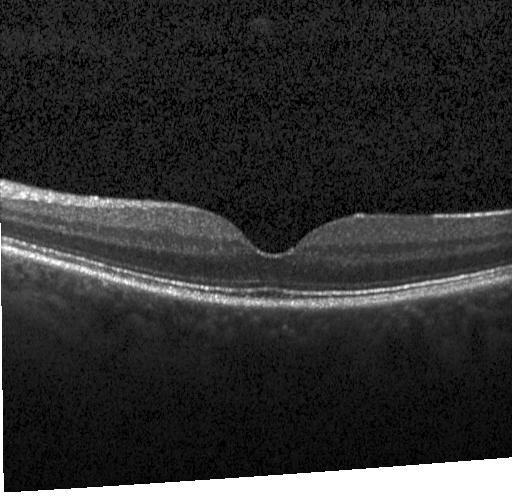
Retinal OCT B-scan · centered on the fovea · SD-OCT · Heidelberg Spectralis — OCT finding: no choroidal neovascularization, no diabetic macular edema, and no drusen.